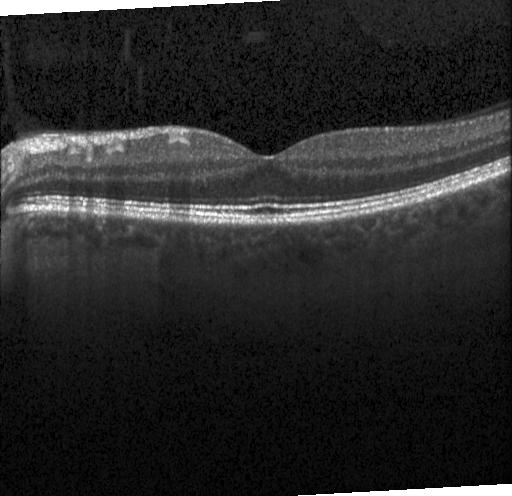
OCT B-scan showing no evidence of choroidal neovascularization, diabetic macular edema, or drusen.